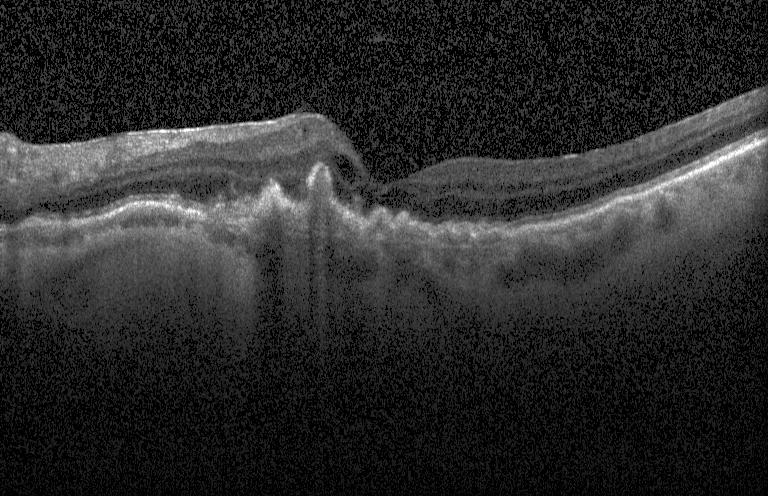

Retinal OCT B-scan
Diagnosis: a choroidal neovascular membrane.